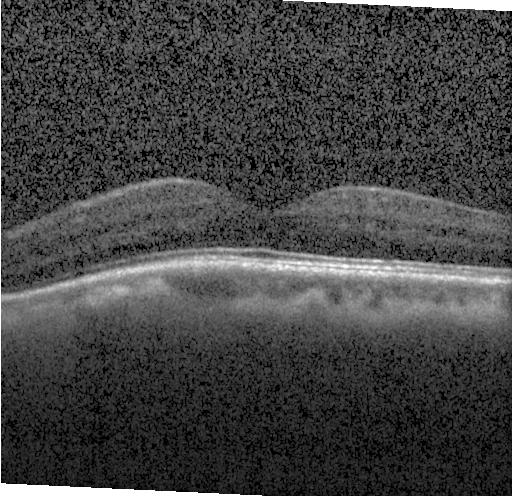
Retinal OCT cross-section showing no choroidal neovascularization, diabetic macular edema, or drusen.